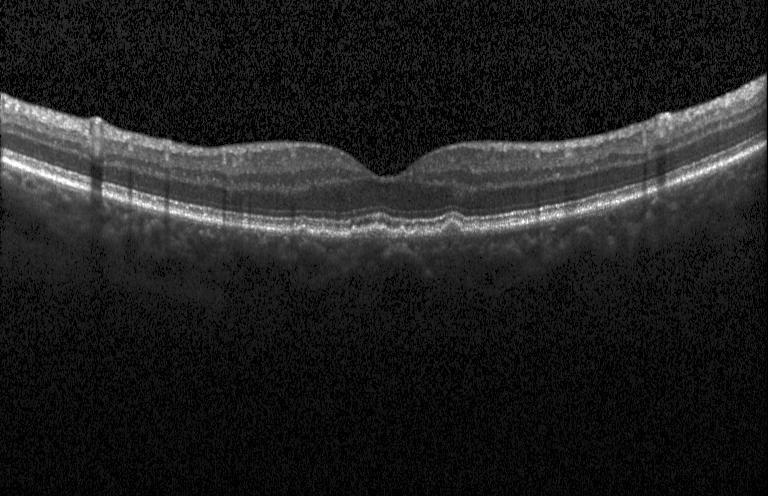

Horizontal scan through the fovea · optical coherence tomography B-scan · spectral-domain optical coherence tomography · instrument: Heidelberg Spectralis
Impression: multiple drusen.